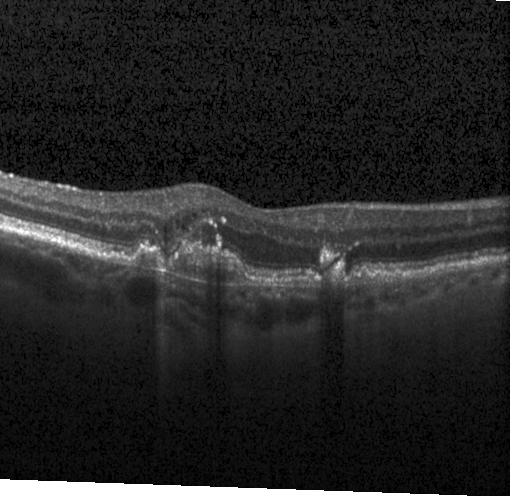

OCT B-scan
Macular OCT: choroidal neovascularization.